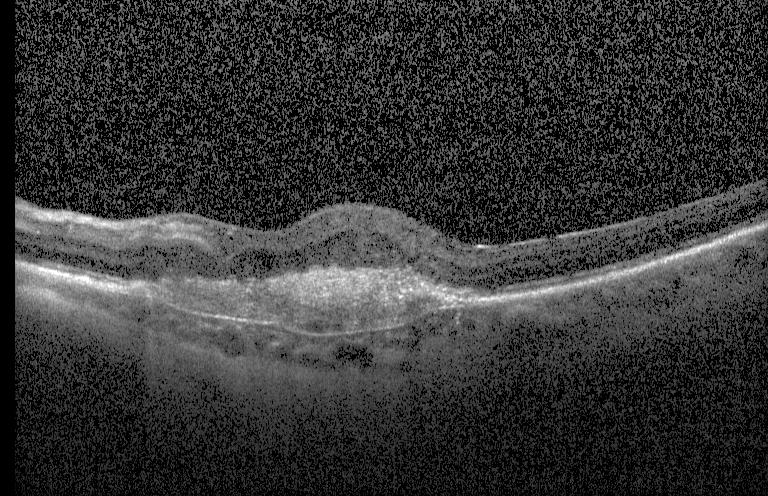
SD-OCT. Heidelberg Spectralis. Optical coherence tomography scan. Finding: a choroidal neovascular membrane.